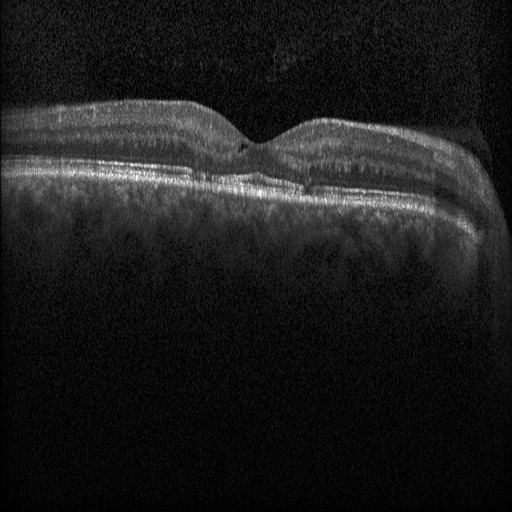

Retinal OCT cross-section, fovea-centered, Heidelberg Spectralis OCT system. Macular OCT: DME.